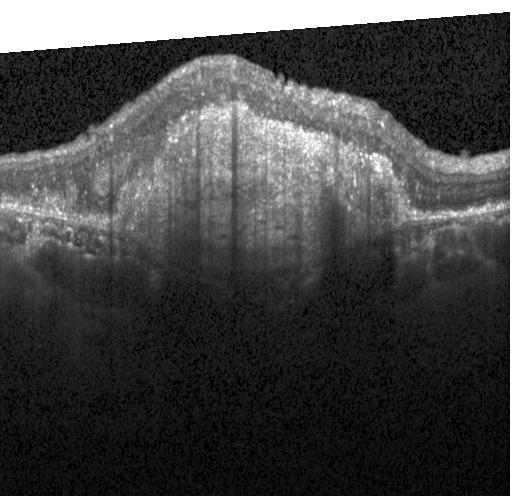
Retinal OCT cross-section. Centered on the fovea. SD-OCT. Instrument: Heidelberg Spectralis.
Finding: CNV.